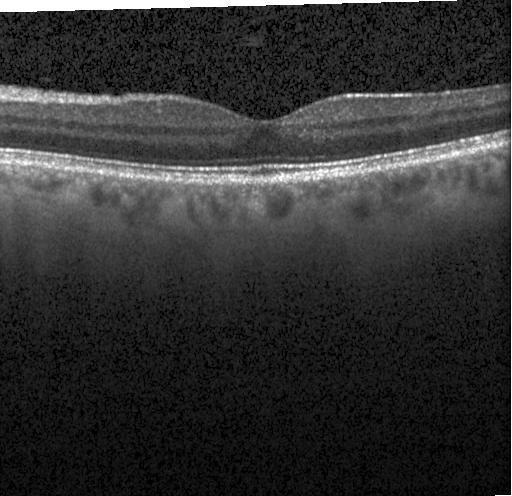
OCT line scan; centered on the fovea. Impression: neither CNV, DME, nor drusen.